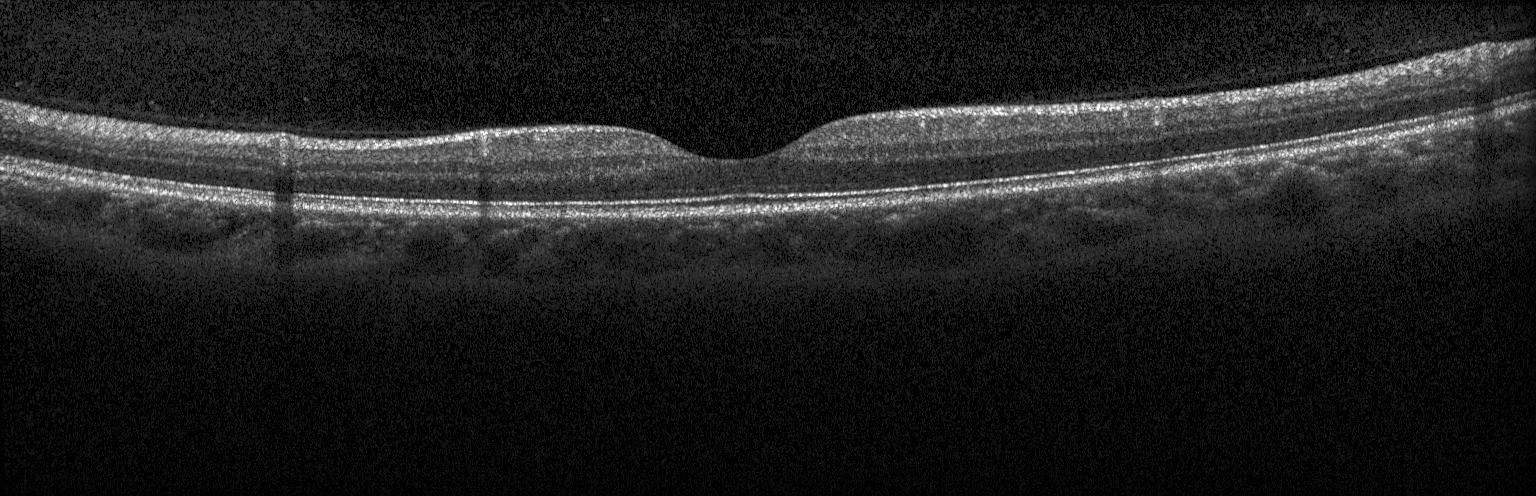 OCT B-scan. Diagnosis: no CNV, no DME, and no drusen.